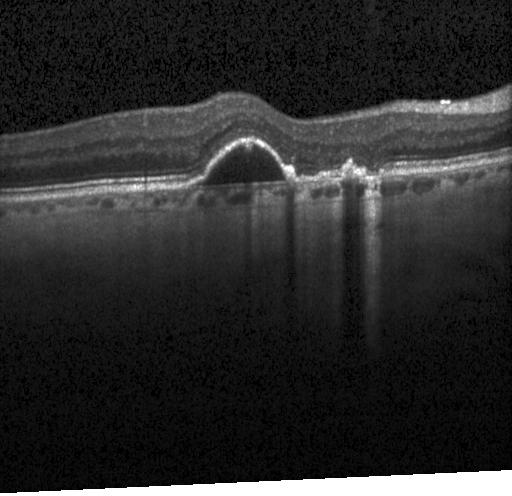
OCT finding: CNV.